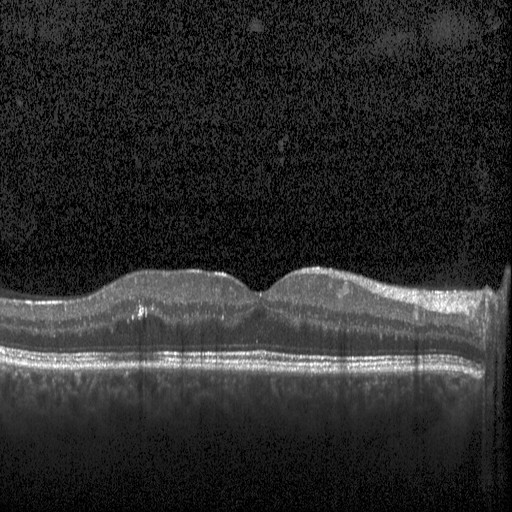

OCT scan showing diabetic macular edema (DME).